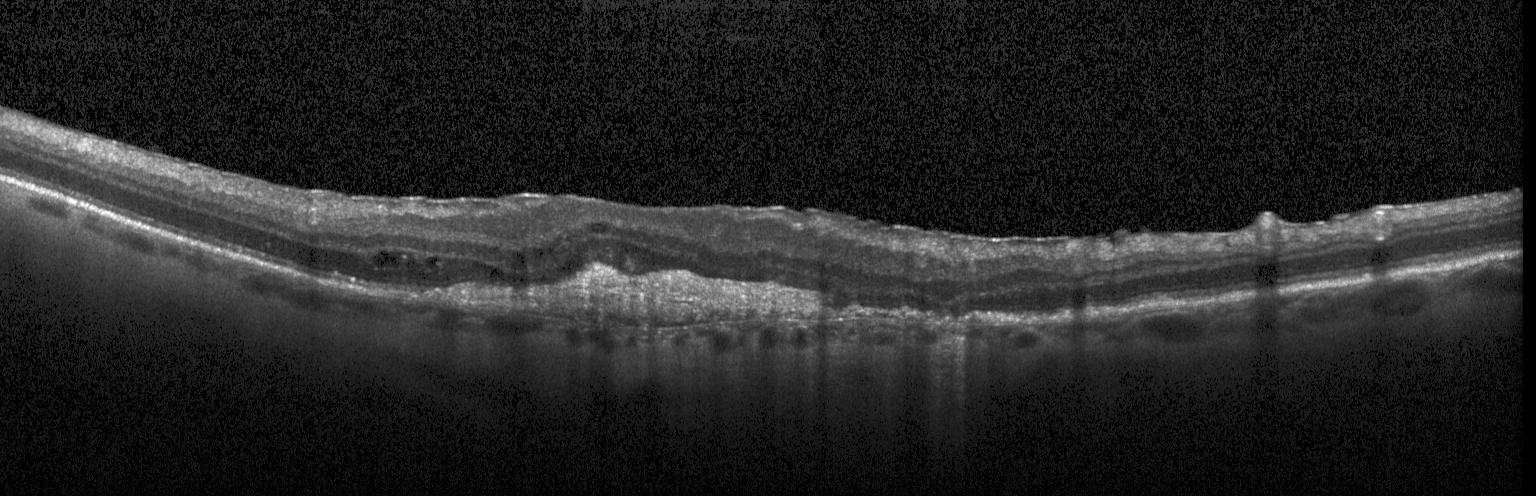
Finding: a choroidal neovascular membrane.